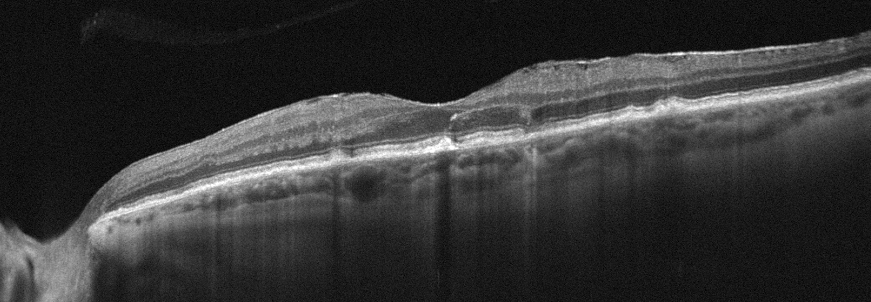

Retinal OCT B-scan. Instrument: Optovue Avanti RTVue XR — Dx: age-related macular degeneration.